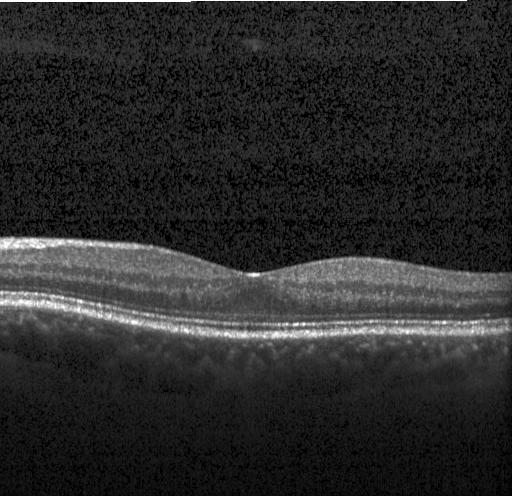
Optical coherence tomography scan; fovea-centered. Macular OCT: no CNV, DME, or drusen.